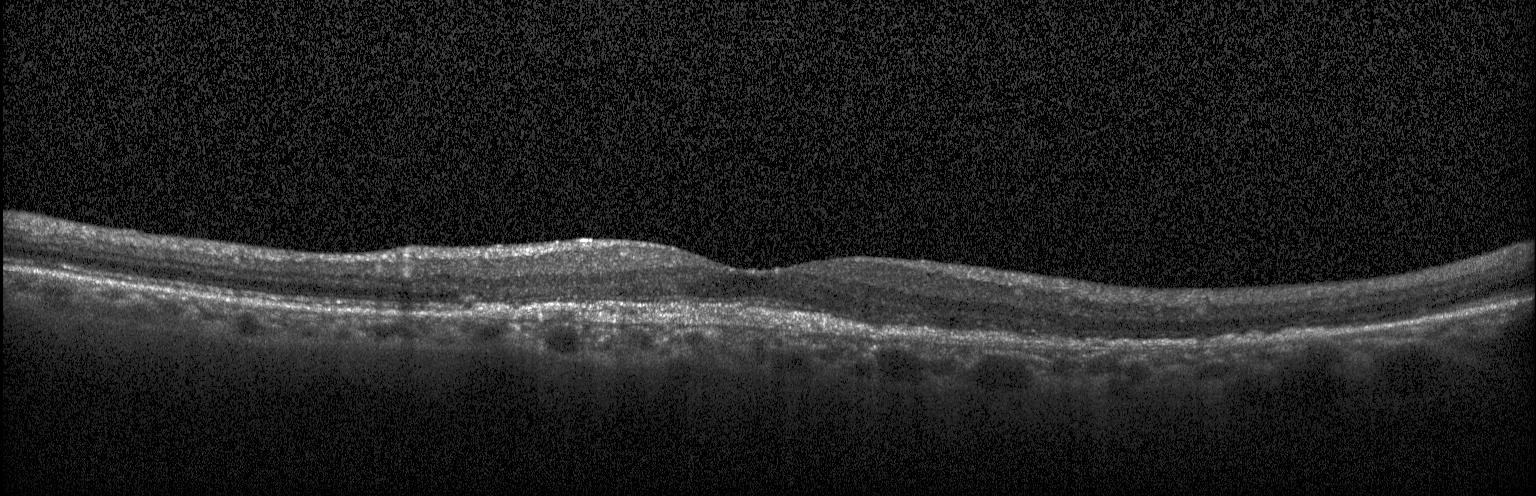

Diagnosis: a choroidal neovascular membrane.